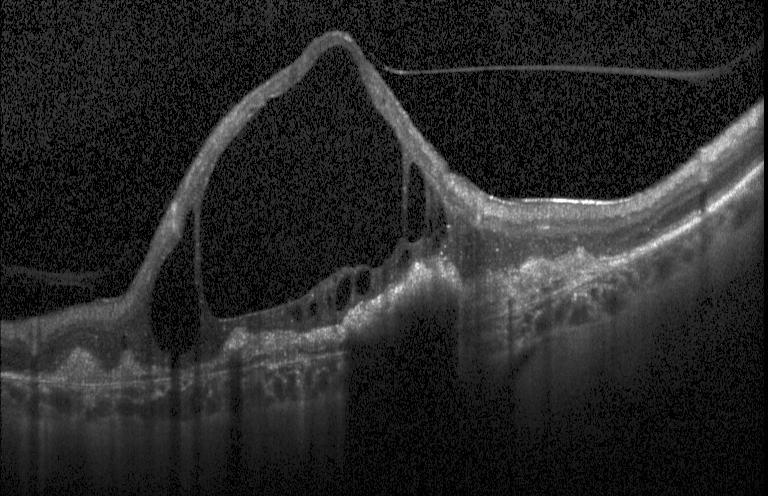
Optical coherence tomography scan · horizontal scan through the fovea.
Finding: a choroidal neovascular membrane.